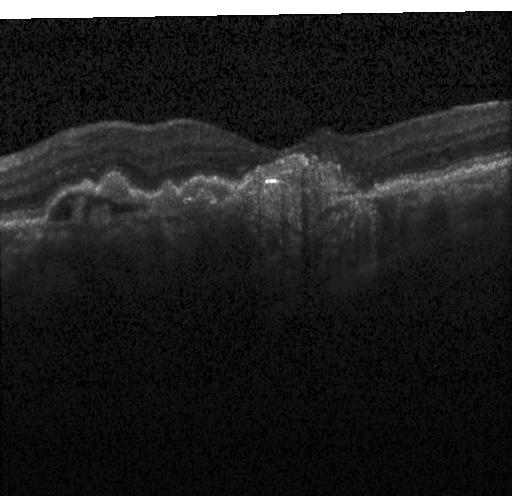
Impression: a choroidal neovascular membrane.